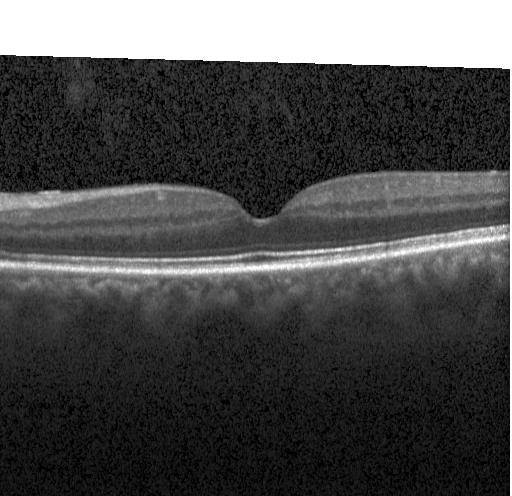

Optical coherence tomography B-scan · instrument: Heidelberg Spectralis · spectral-domain optical coherence tomography. This B-scan demonstrates no evidence of choroidal neovascularization, diabetic macular edema, or drusen.